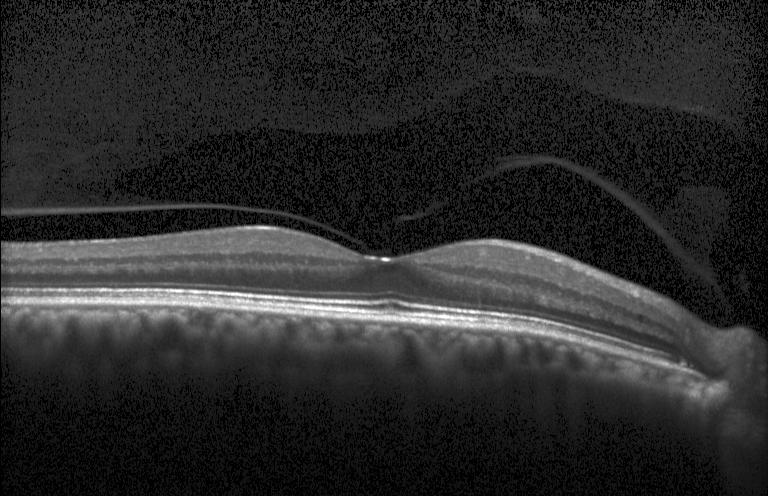

Dx: no choroidal neovascularization, no diabetic macular edema, and no drusen.